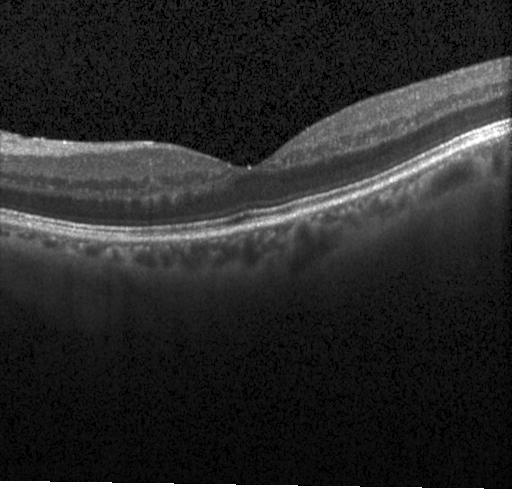

OCT scan showing no evidence of choroidal neovascularization, diabetic macular edema, or drusen.